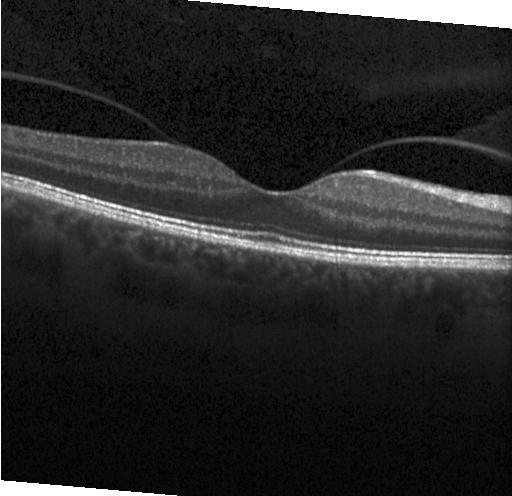
Heidelberg Spectralis OCT system · spectral-domain OCT · OCT B-scan · horizontal scan through the fovea
Dx: neither choroidal neovascularization, diabetic macular edema, nor drusen.